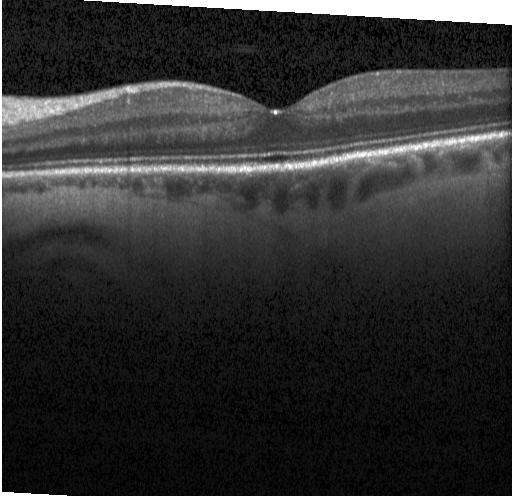 OCT B-scan
Assessment: no CNV, no DME, and no drusen.